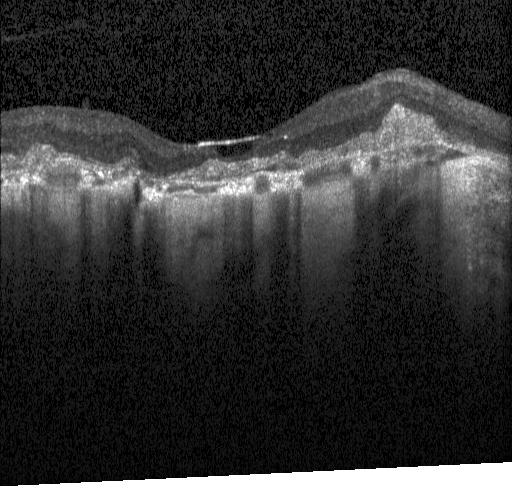 OCT B-scan. Instrument: Heidelberg Spectralis. Diagnosis: choroidal neovascularization (CNV).